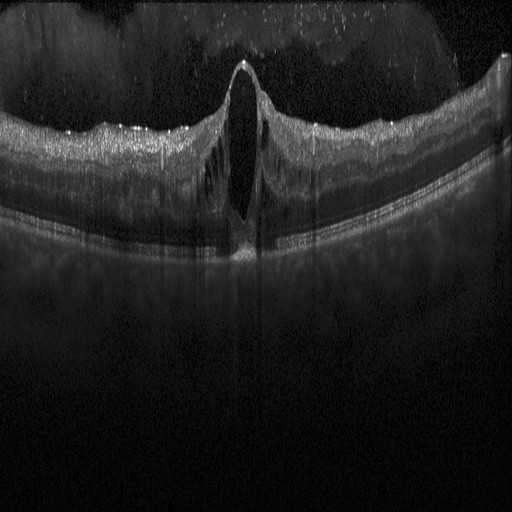
Fovea-centered · optical coherence tomography B-scan — Macular OCT: DME.